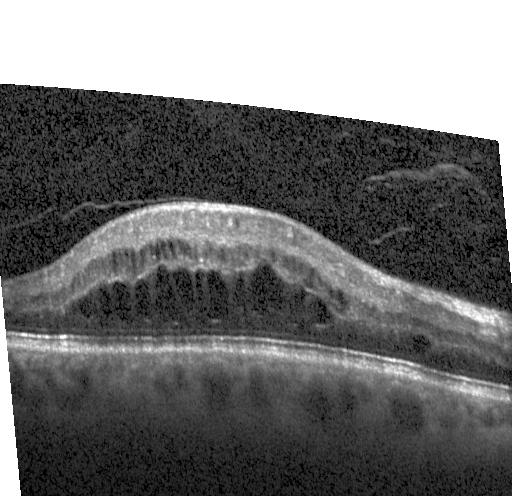

Centered on the fovea. Optical coherence tomography B-scan. Impression: diabetic macular edema.